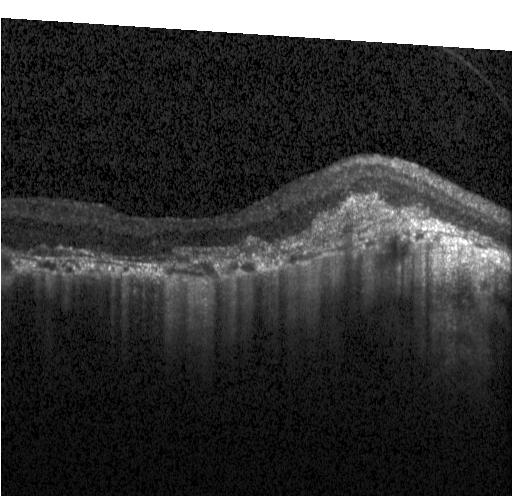 Heidelberg Spectralis OCT system, optical coherence tomography scan, spectral-domain OCT
Impression: CNV.